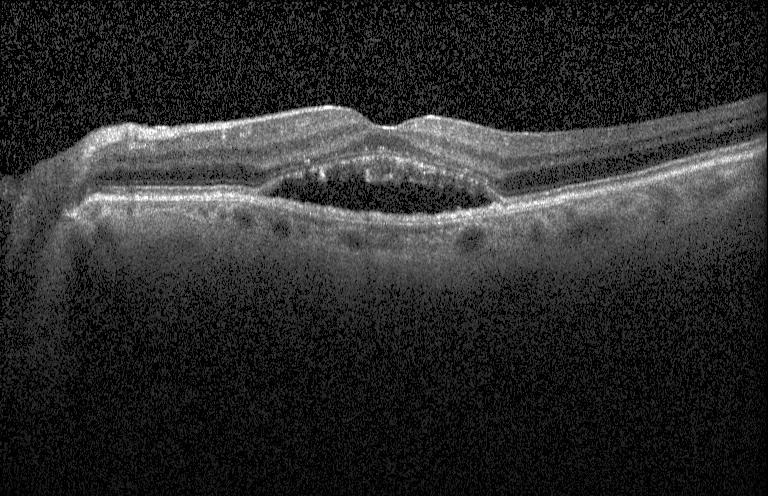
Assessment: choroidal neovascularization.